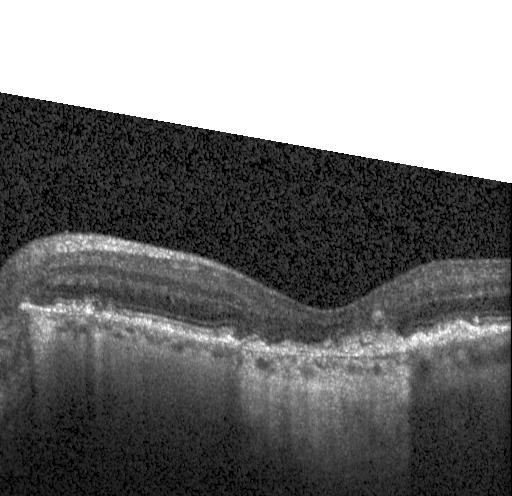
A choroidal neovascular membrane.